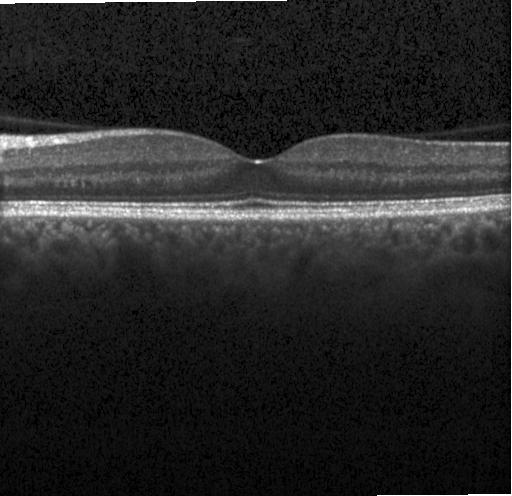
OCT B-scan showing no CNV, DME, or drusen.